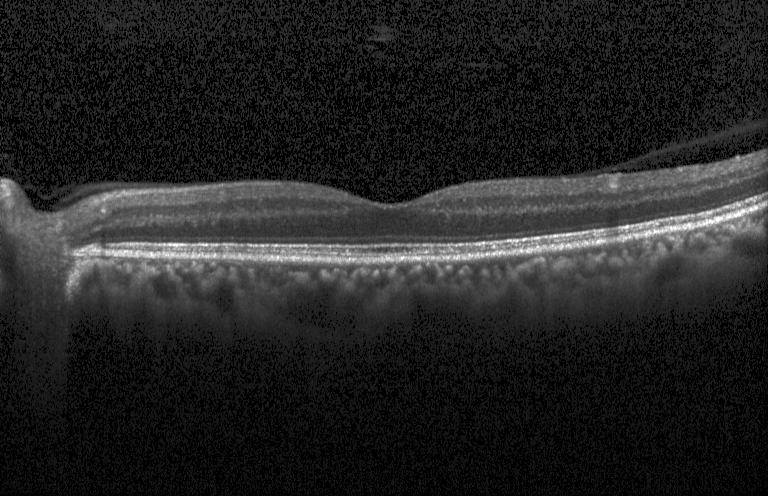

Optical coherence tomography B-scan.
Finding: neither choroidal neovascularization, diabetic macular edema, nor drusen.